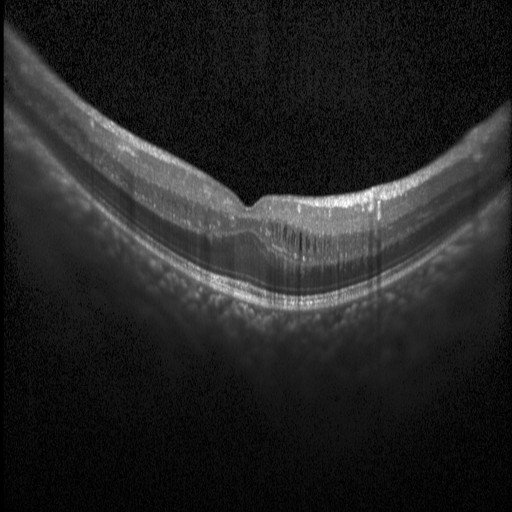
OCT line scan, Heidelberg Spectralis OCT system, horizontal scan through the fovea — Diabetic macular edema.